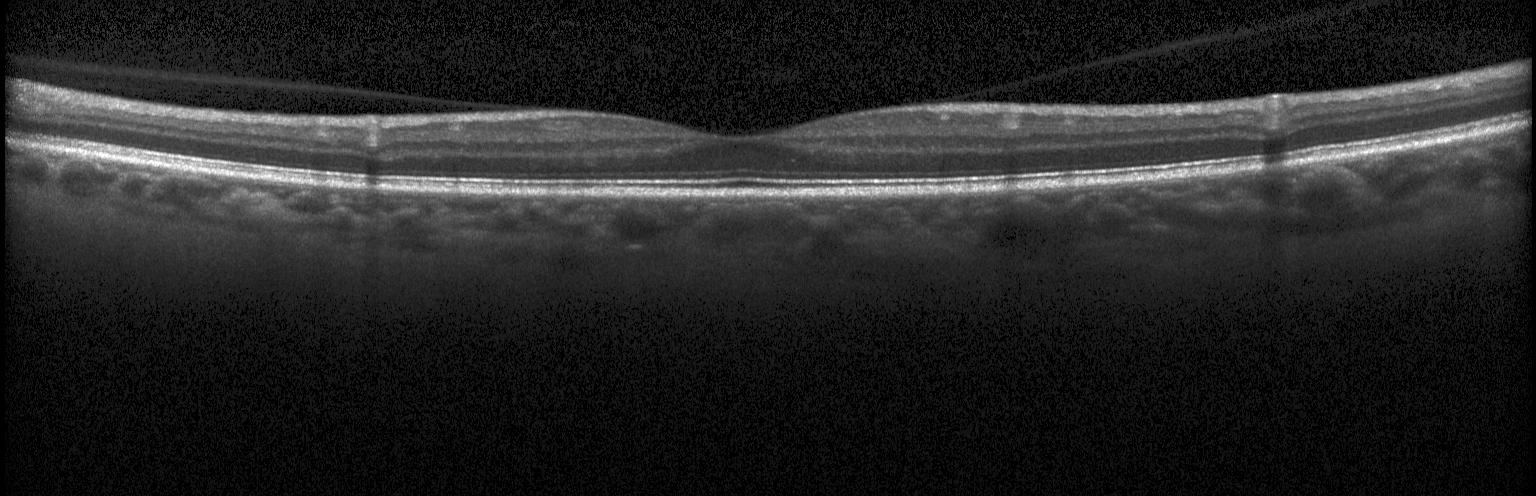 Fovea-centered; OCT B-scan; instrument: Heidelberg Spectralis; spectral-domain optical coherence tomography — This B-scan demonstrates neither choroidal neovascularization, diabetic macular edema, nor drusen.